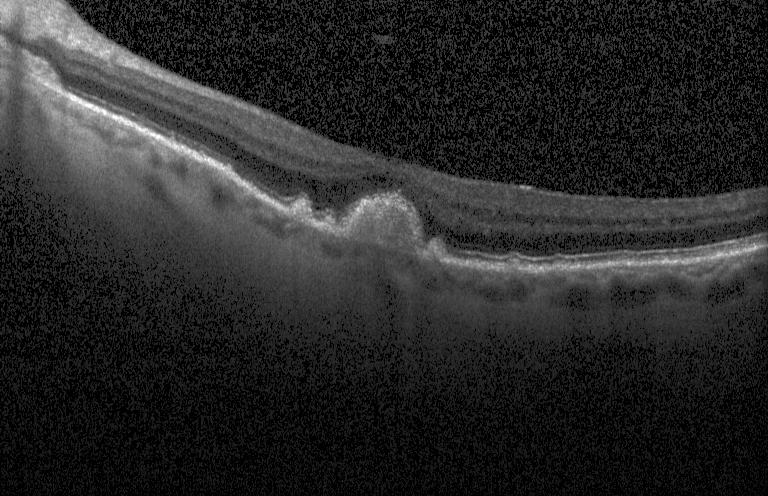
The scan shows sub-RPE drusenoid deposits.